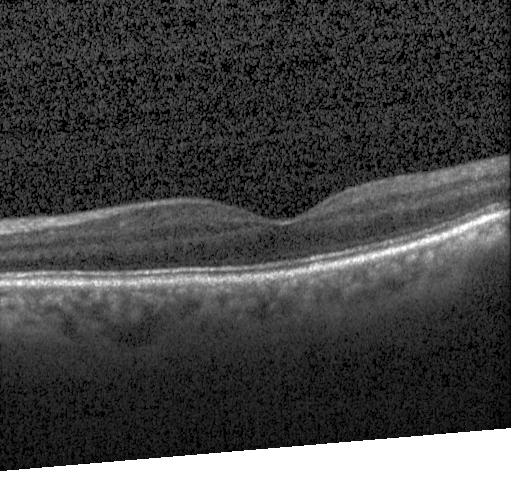
Acquired on a Heidelberg Spectralis. SD-OCT. Through the macula. Retinal OCT B-scan
This B-scan demonstrates neither CNV, DME, nor drusen.